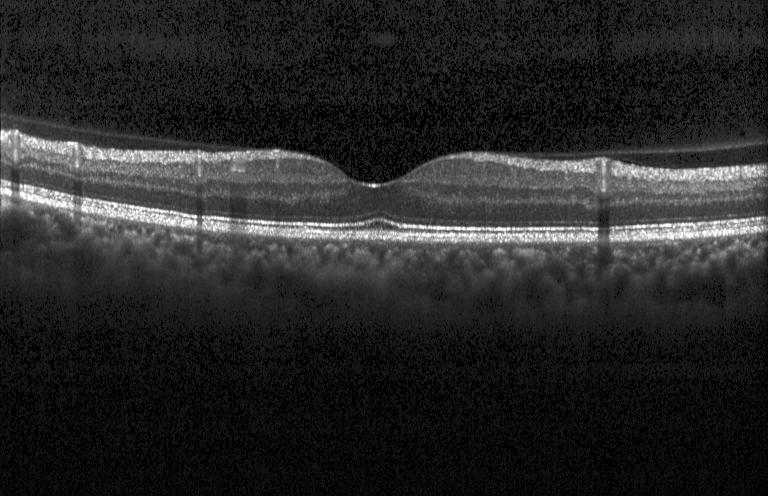
Through the macula. OCT line scan. Heidelberg Spectralis.
Finding: no evidence of CNV, DME, or drusen.